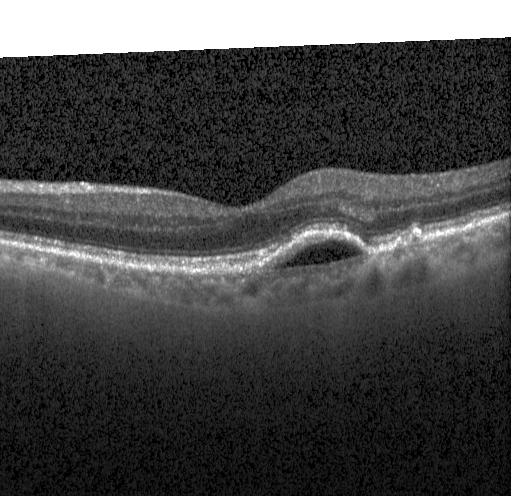

Impression: choroidal neovascularization (CNV).